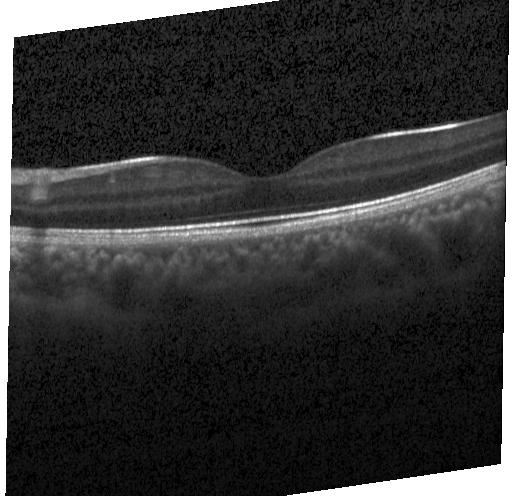

Diagnosis: no choroidal neovascularization, diabetic macular edema, or drusen.